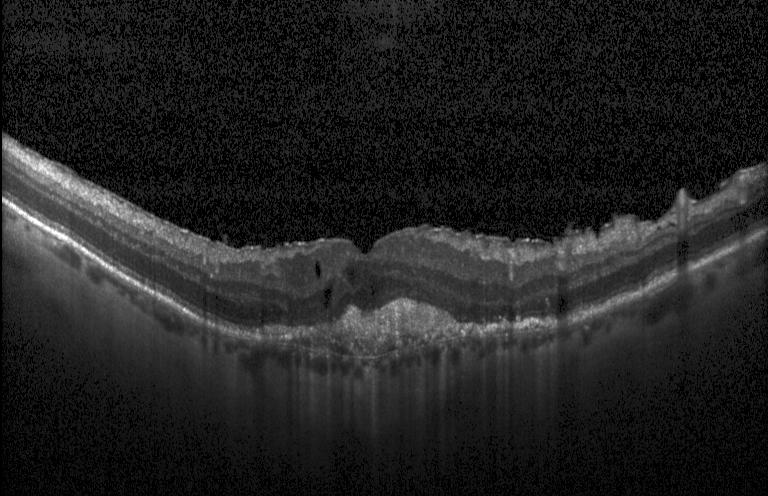
Optical coherence tomography scan. Heidelberg Spectralis — Impression: CNV.